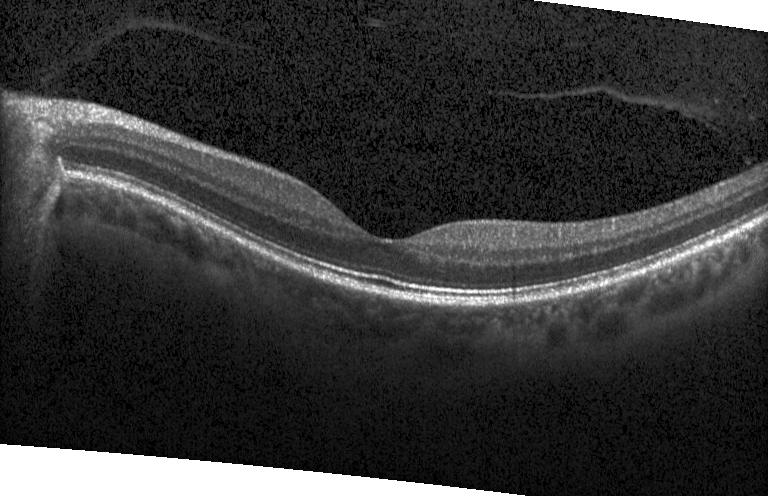

Assessment: no evidence of CNV, DME, or drusen.